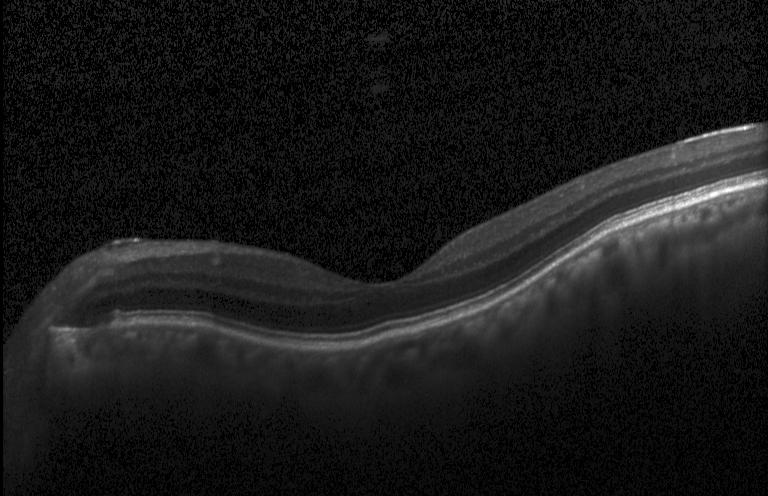 Impression: no choroidal neovascularization, diabetic macular edema, or drusen.